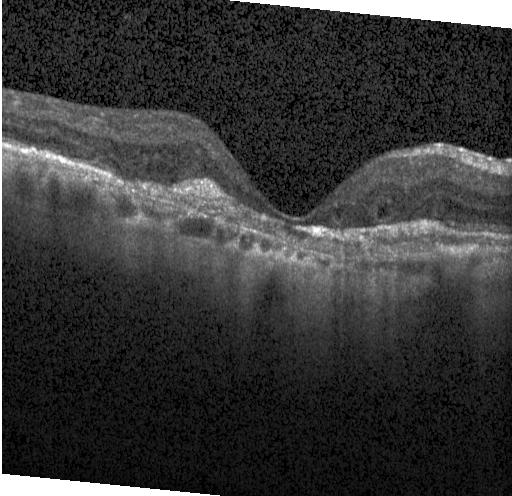
Retinal OCT cross-section; through the macula — Choroidal neovascularization (CNV).